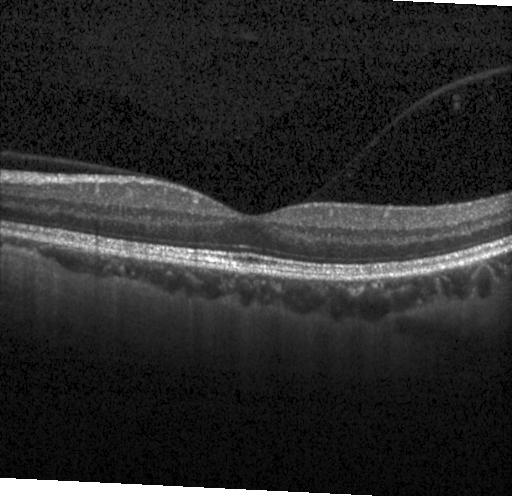 Instrument: Heidelberg Spectralis; OCT line scan — Dx: no choroidal neovascularization, diabetic macular edema, or drusen.